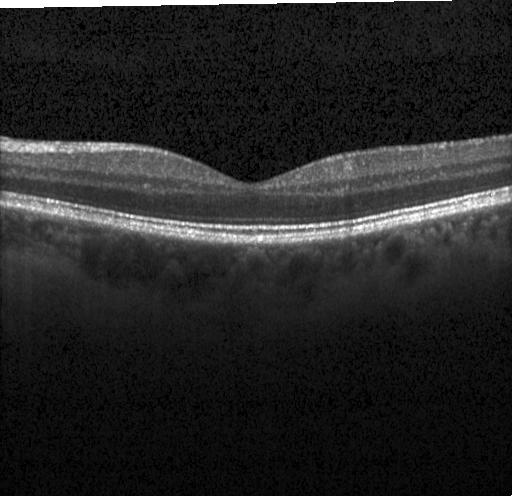 Retinal OCT cross-section. Impression: no evidence of CNV, DME, or drusen.